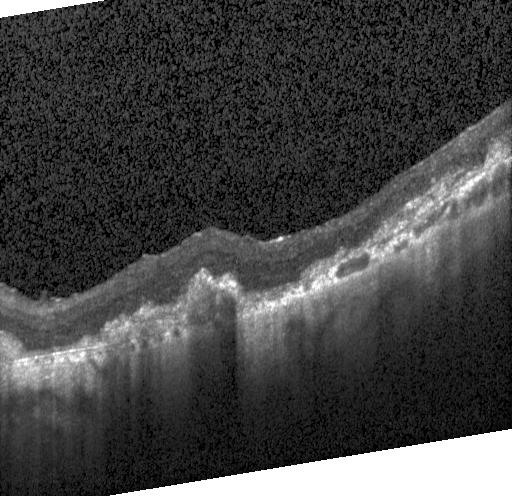

Finding: choroidal neovascularization.